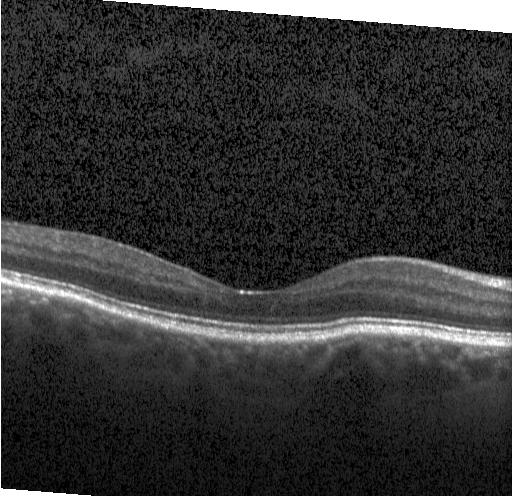 Impression: neither choroidal neovascularization, diabetic macular edema, nor drusen.